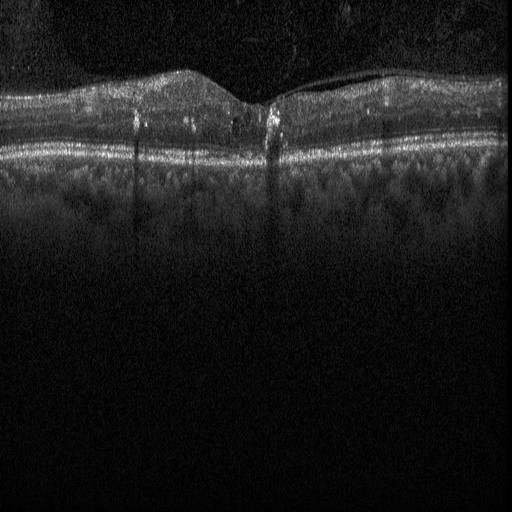

Macular scan, optical coherence tomography B-scan, acquired on a Heidelberg Spectralis, SD-OCT — Impression: diabetic macular edema.